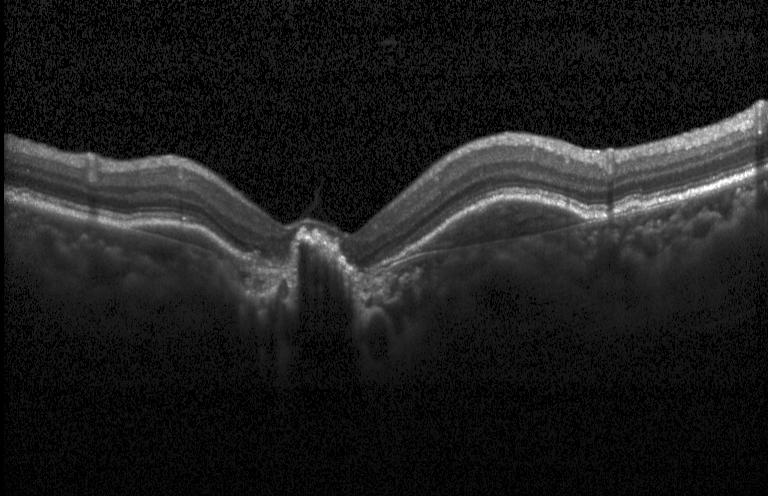

OCT B-scan showing a choroidal neovascular membrane.